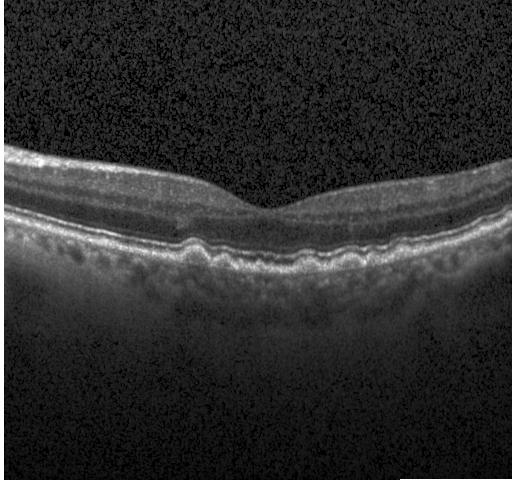

The scan shows sub-RPE drusenoid deposits.